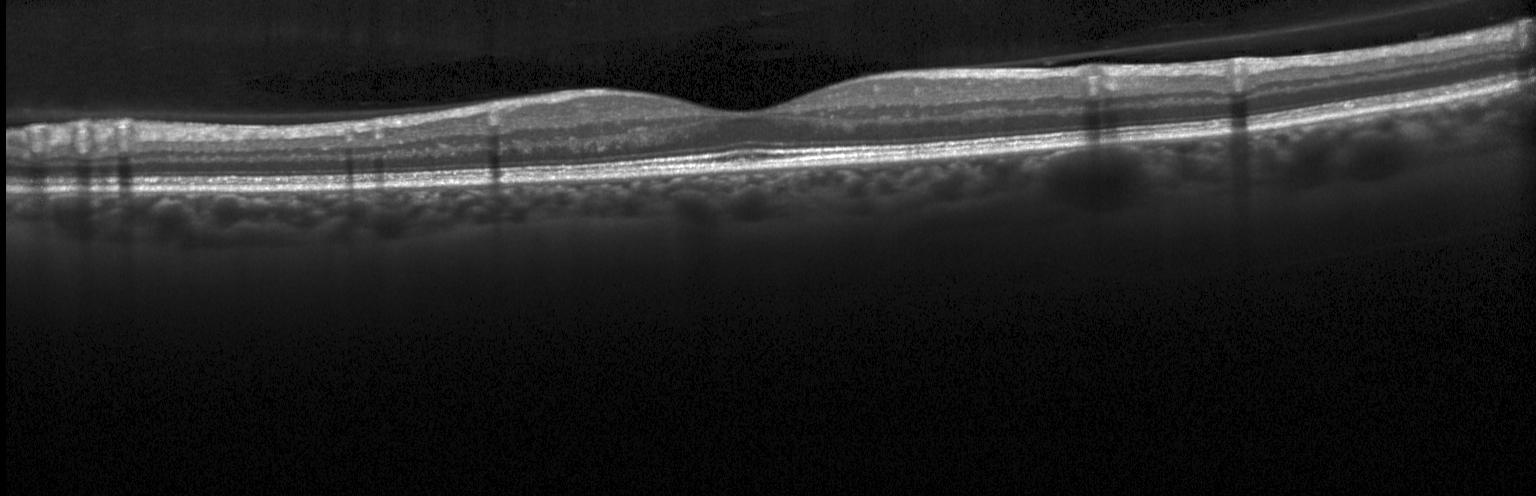

Retinal OCT B-scan
Finding: no CNV, DME, or drusen.